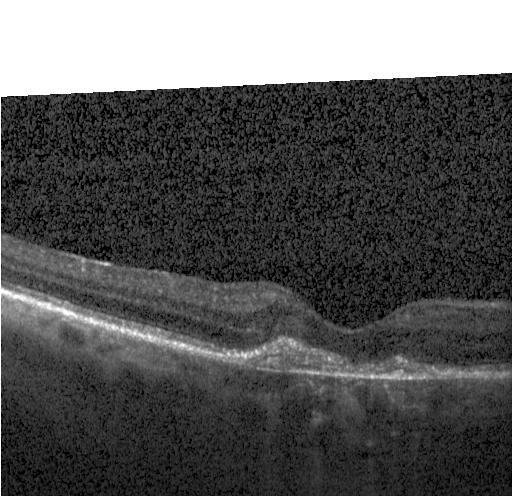

Finding: CNV.